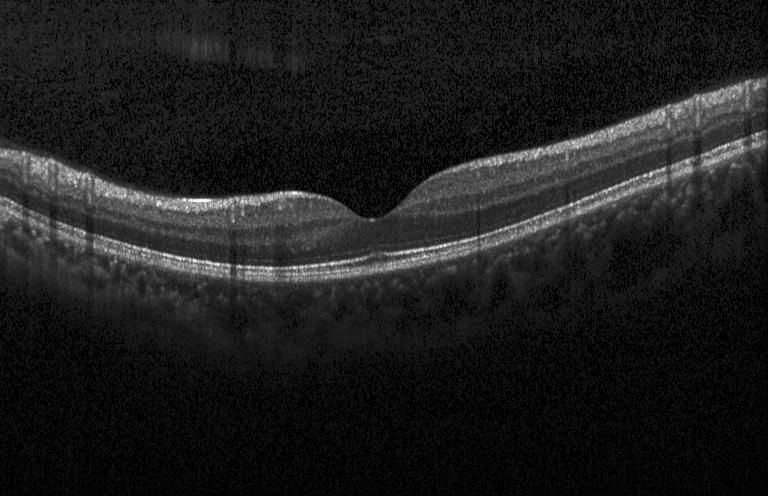
Macular OCT demonstrating no evidence of choroidal neovascularization, diabetic macular edema, or drusen.